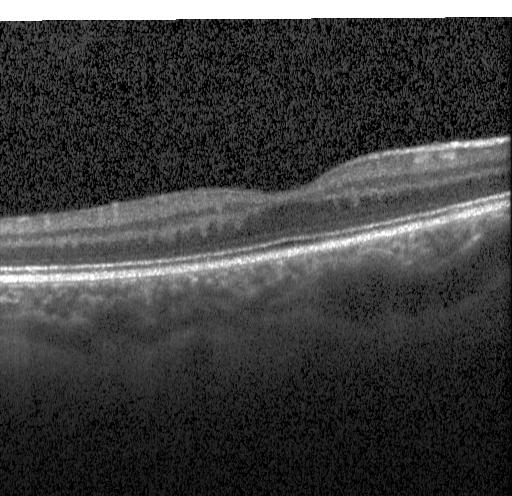 Diagnosis: neither choroidal neovascularization, diabetic macular edema, nor drusen.